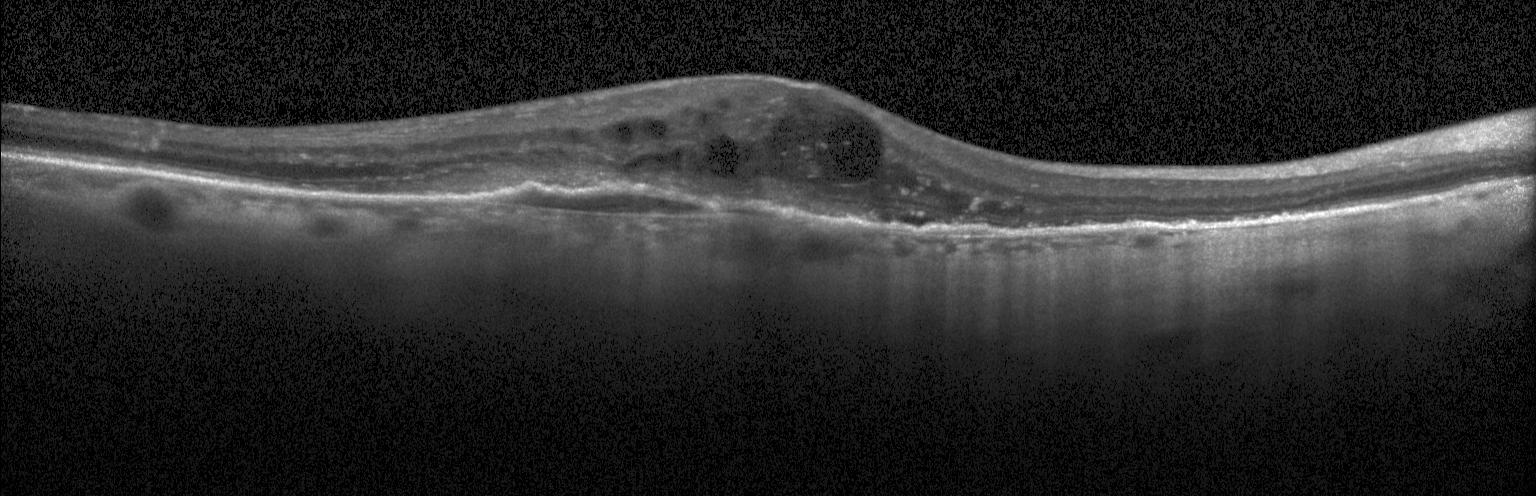
OCT B-scan. Diagnosis: choroidal neovascularization.